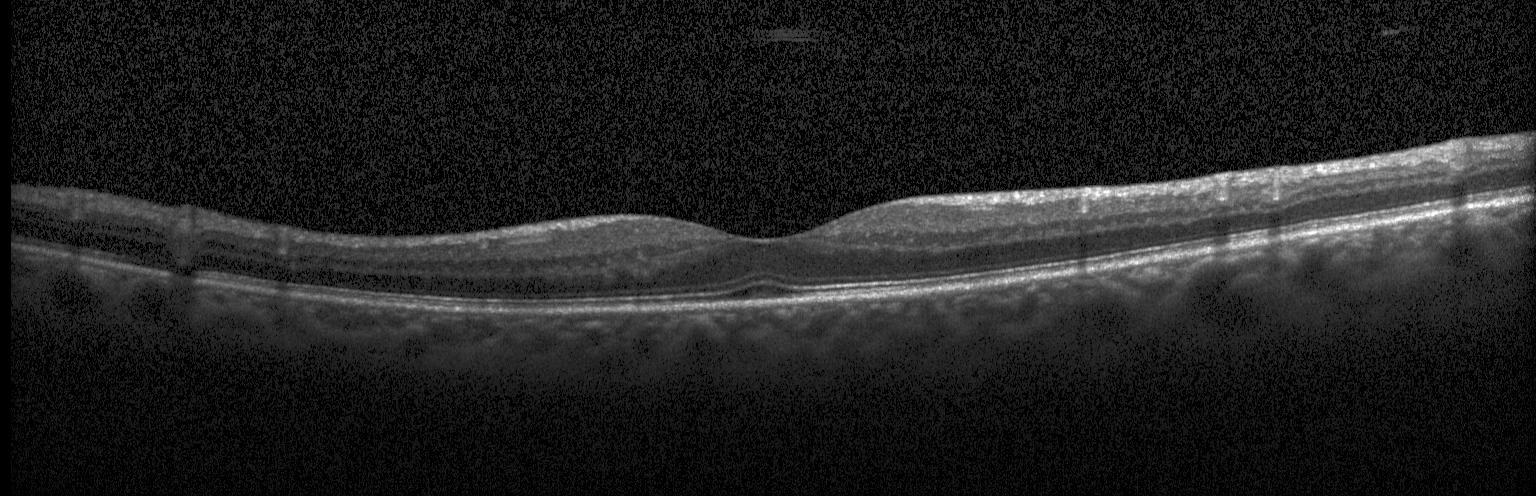

Optical coherence tomography scan — Macular OCT: no choroidal neovascularization, no diabetic macular edema, and no drusen.